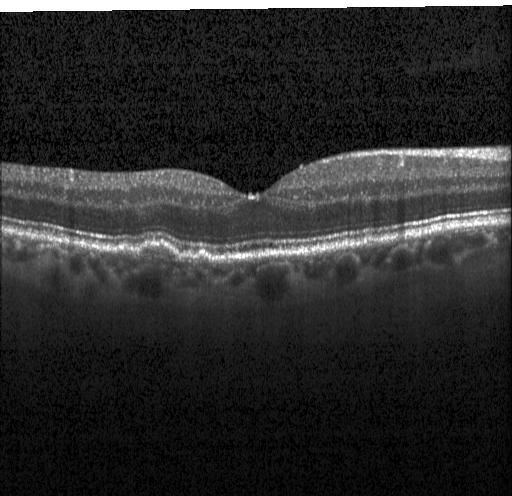
Fovea-centered, OCT line scan, spectral-domain OCT. Impression: sub-RPE drusenoid deposits.